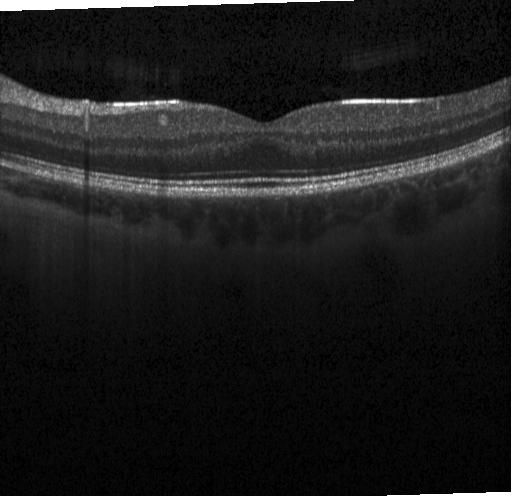 Optical coherence tomography scan. Impression: no CNV, DME, or drusen.